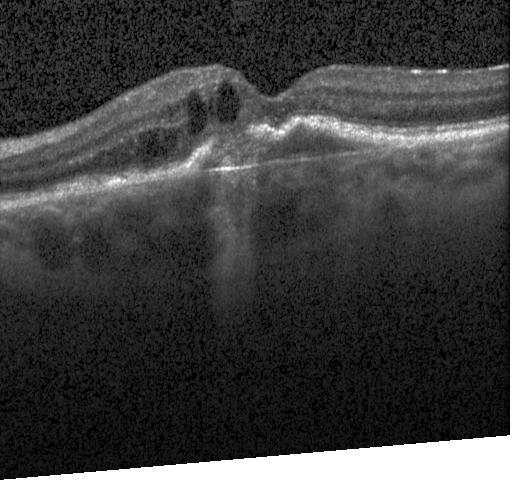

Heidelberg Spectralis OCT system · optical coherence tomography scan.
The scan shows choroidal neovascularization (CNV).